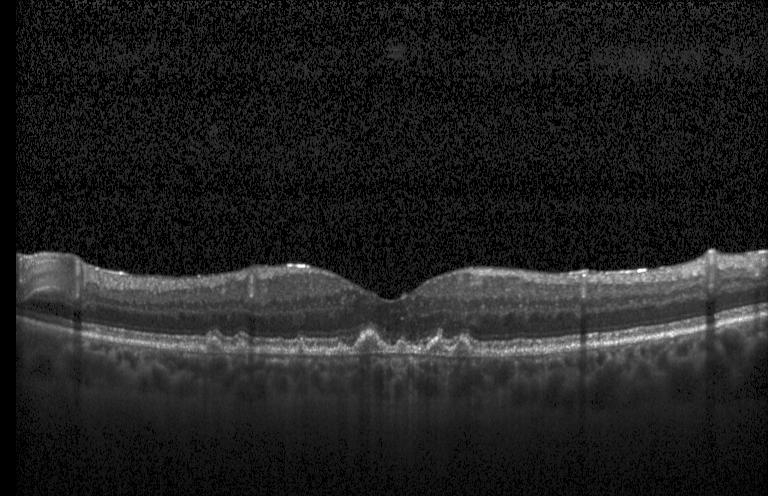
Optical coherence tomography scan, Heidelberg Spectralis OCT system, fovea-centered, spectral-domain optical coherence tomography.
Diagnosis: multiple drusen.